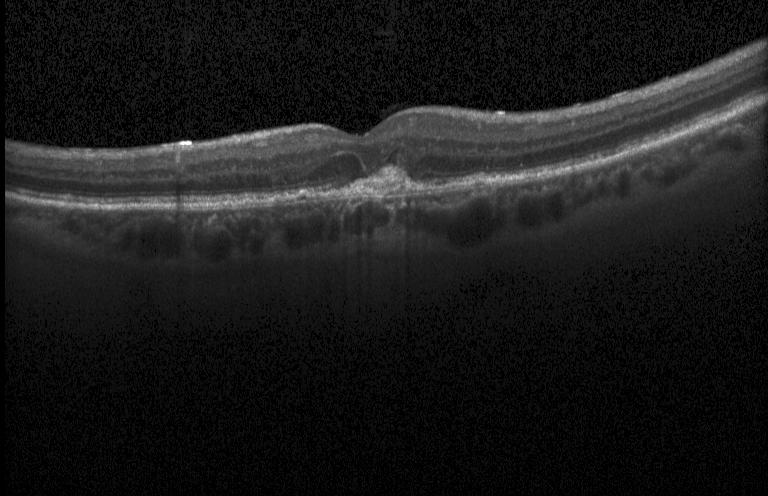

OCT B-scan
This B-scan demonstrates a choroidal neovascular membrane.